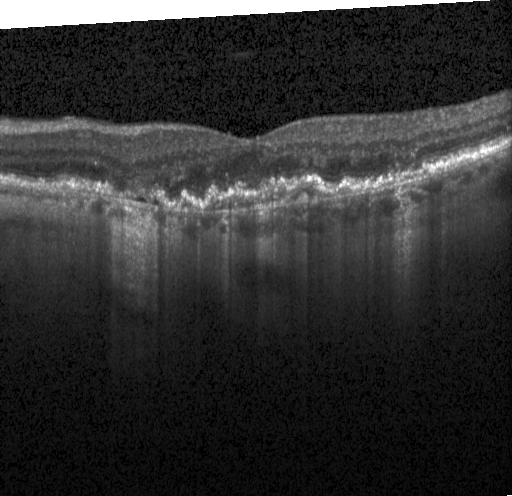

Fovea-centered, SD-OCT, OCT B-scan
Dx: choroidal neovascularization.